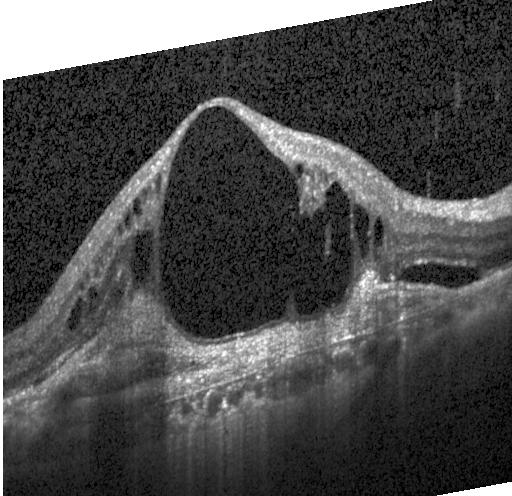
This B-scan demonstrates a choroidal neovascular membrane.